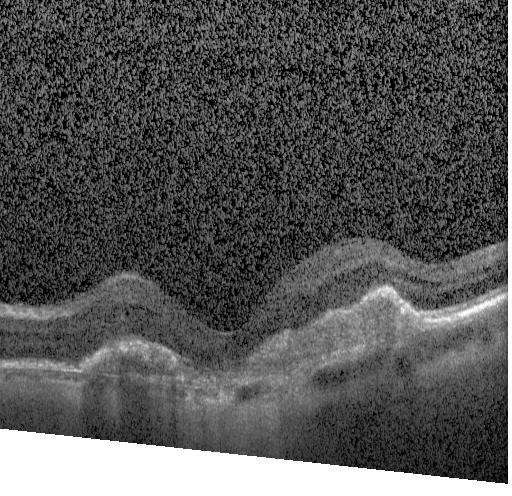
Instrument: Heidelberg Spectralis, SD-OCT, OCT line scan
OCT finding: a choroidal neovascular membrane.